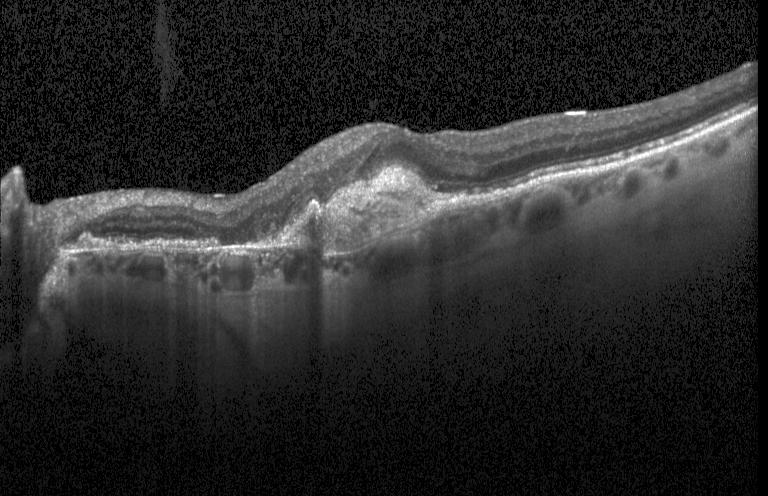

OCT line scan. Heidelberg Spectralis. Spectral-domain OCT. Centered on the fovea.
Diagnosis: a choroidal neovascular membrane.